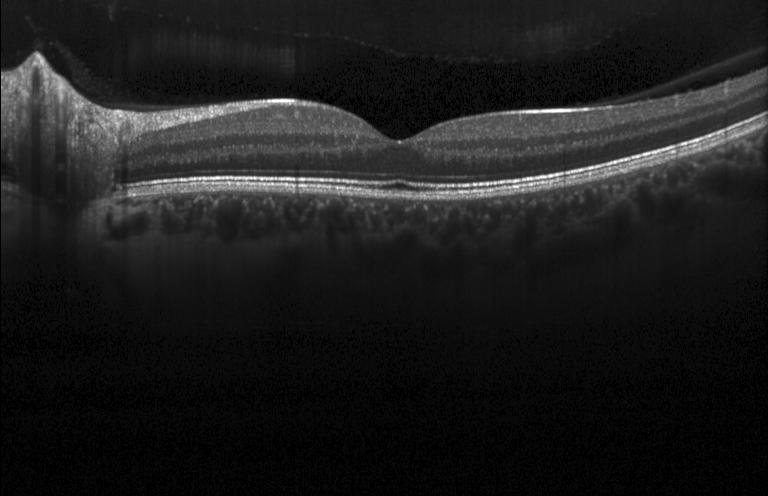 OCT line scan, instrument: Heidelberg Spectralis, horizontal scan through the fovea, spectral-domain optical coherence tomography. No choroidal neovascularization, diabetic macular edema, or drusen.